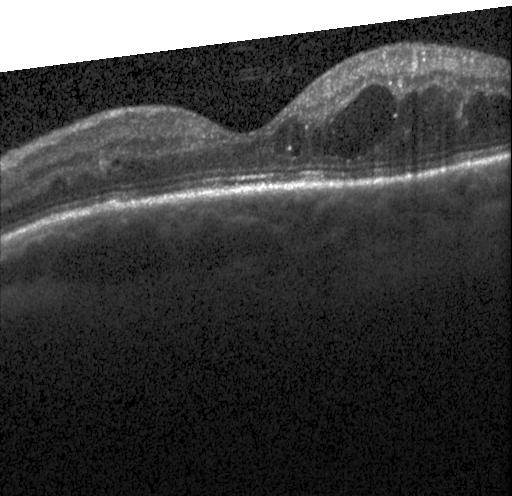

Macular OCT: diabetic macular edema (DME).